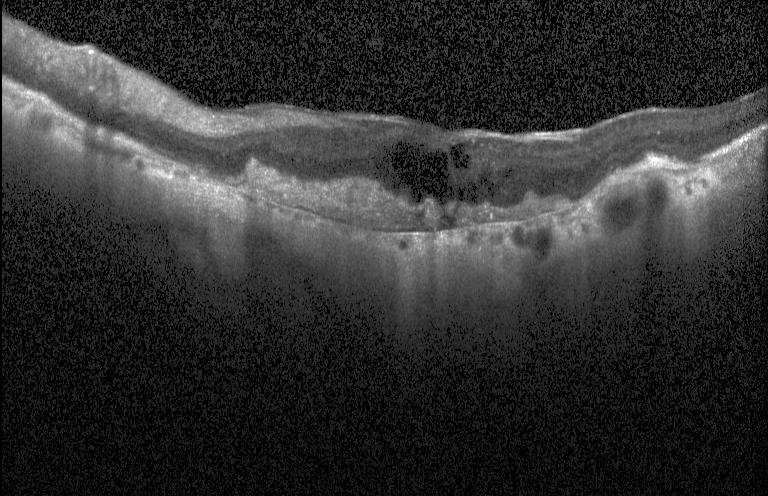
Impression: choroidal neovascularization.